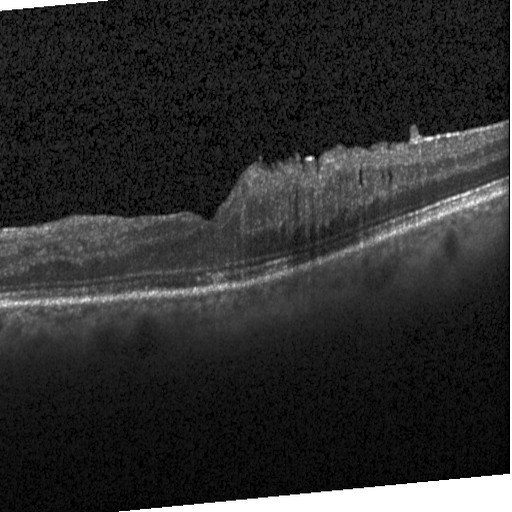

Instrument: Heidelberg Spectralis · spectral-domain optical coherence tomography · retinal OCT B-scan · horizontal scan through the fovea. This B-scan demonstrates diabetic macular edema (DME).